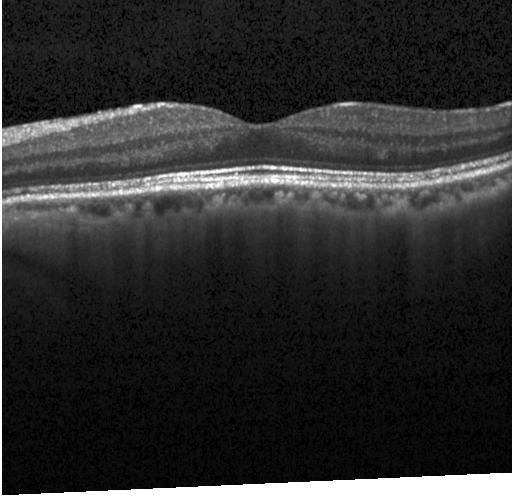

The scan shows no choroidal neovascularization, diabetic macular edema, or drusen.